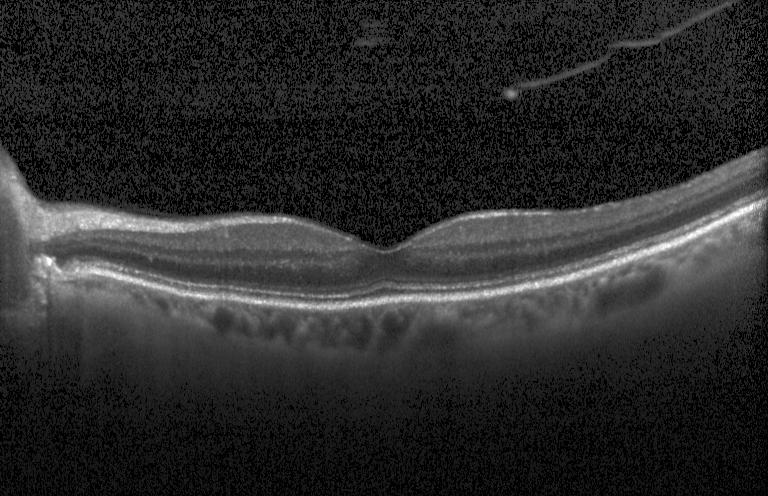 Optical coherence tomography scan — This B-scan demonstrates no choroidal neovascularization, no diabetic macular edema, and no drusen.